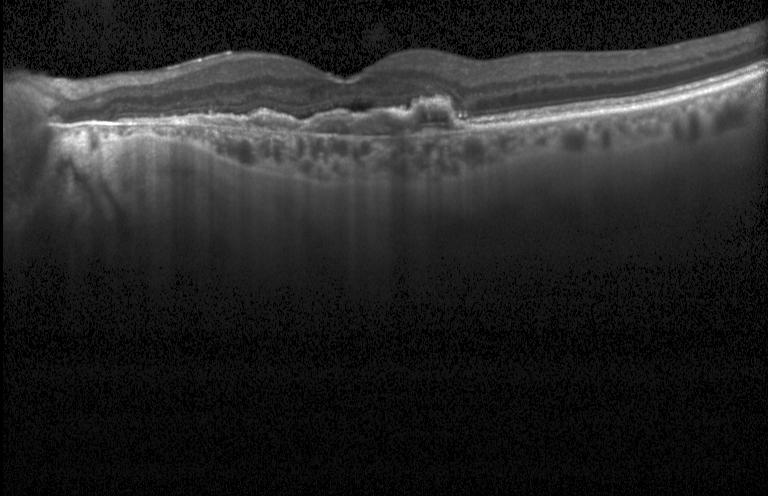
Optical coherence tomography scan.
This B-scan demonstrates a choroidal neovascular membrane.